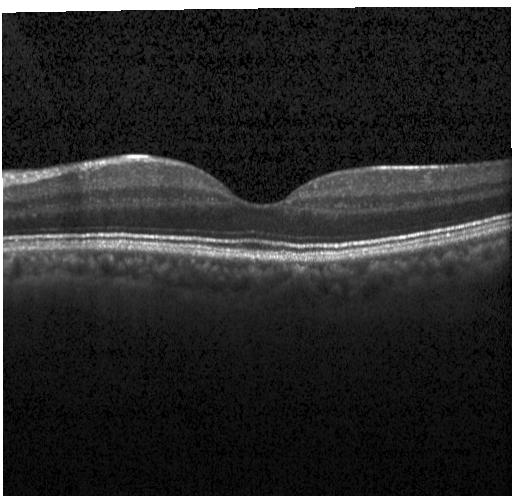 Macular OCT: neither choroidal neovascularization, diabetic macular edema, nor drusen.